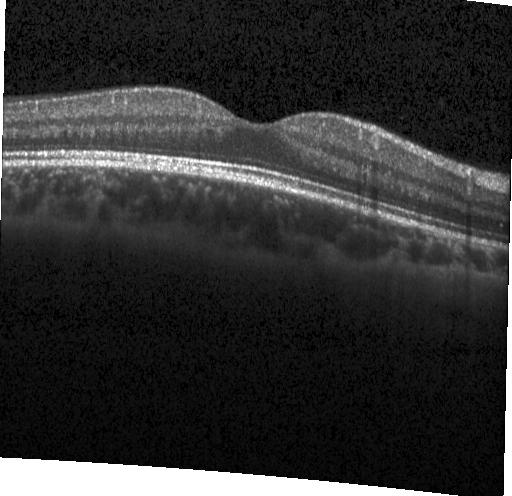 Fovea-centered, spectral-domain OCT, OCT line scan.
Diagnosis: neither CNV, DME, nor drusen.